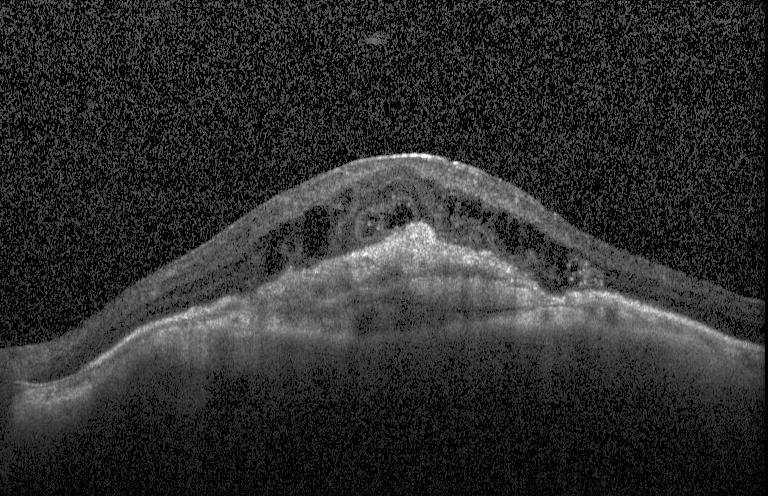 Optical coherence tomography B-scan · through the macula. The scan shows a choroidal neovascular membrane.